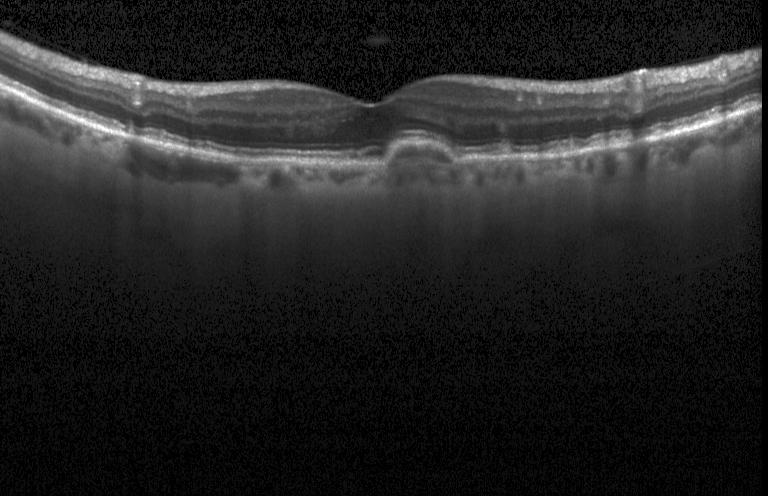

Retinal OCT cross-section, SD-OCT — OCT finding: multiple drusen.